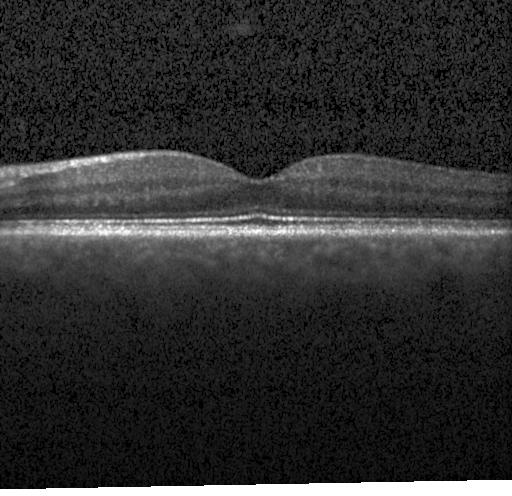 Horizontal scan through the fovea · optical coherence tomography scan · SD-OCT · Heidelberg Spectralis OCT system — Diagnosis: neither CNV, DME, nor drusen.